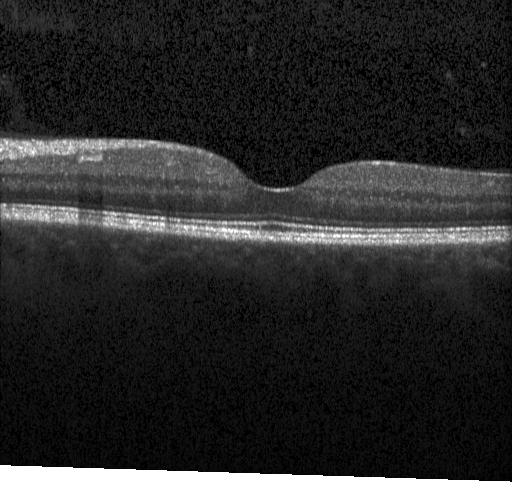
Spectral-domain OCT. Optical coherence tomography B-scan.
Macular OCT: no CNV, no DME, and no drusen.